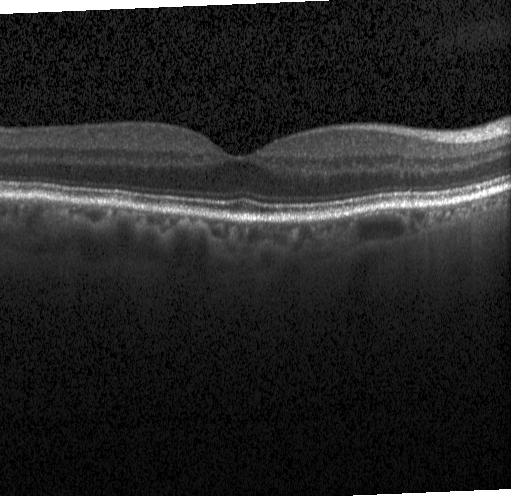

Impression: no evidence of choroidal neovascularization, diabetic macular edema, or drusen.